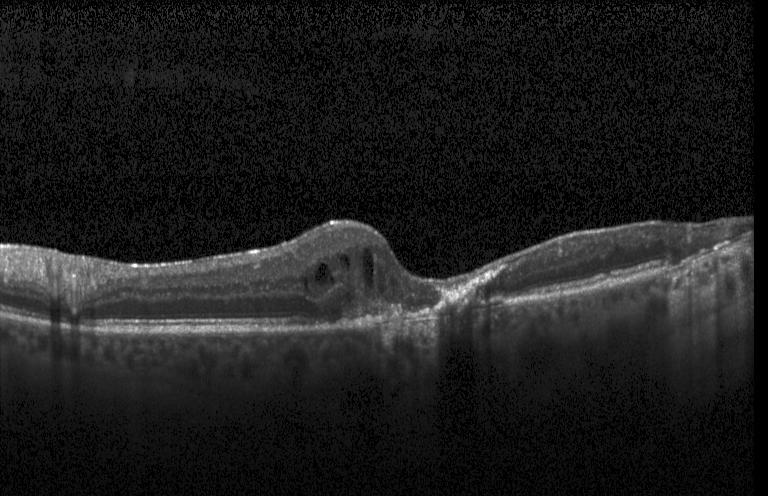
Impression: a choroidal neovascular membrane.